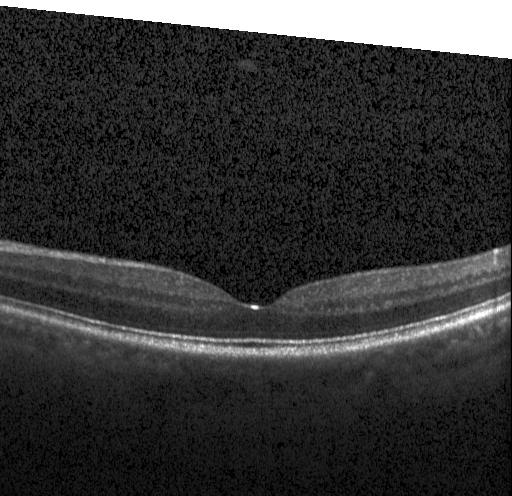
Spectral-domain OCT. Optical coherence tomography B-scan.
Impression: neither choroidal neovascularization, diabetic macular edema, nor drusen.